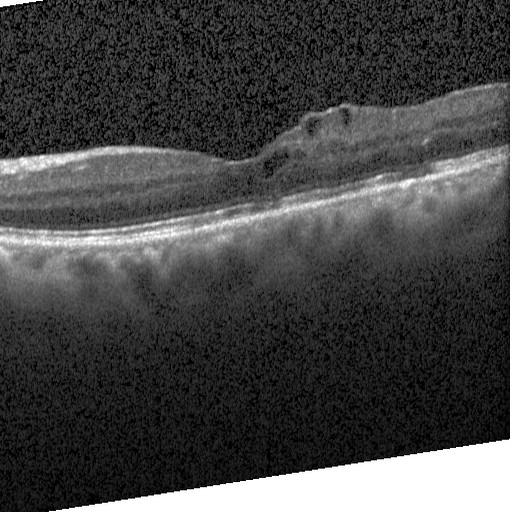 Acquired on a Heidelberg Spectralis, optical coherence tomography B-scan
Diabetic macular edema (DME).